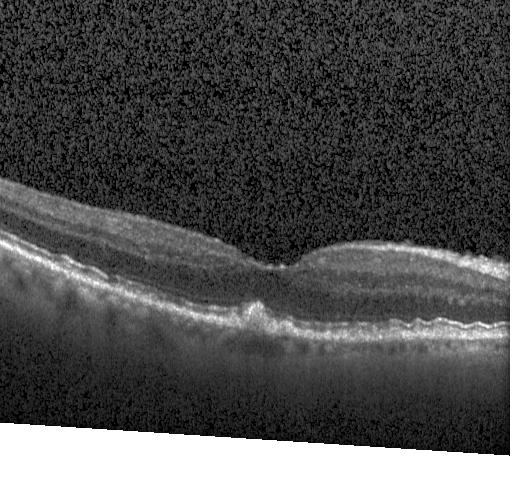 Instrument: Heidelberg Spectralis · spectral-domain OCT · optical coherence tomography scan — Finding: drusen.